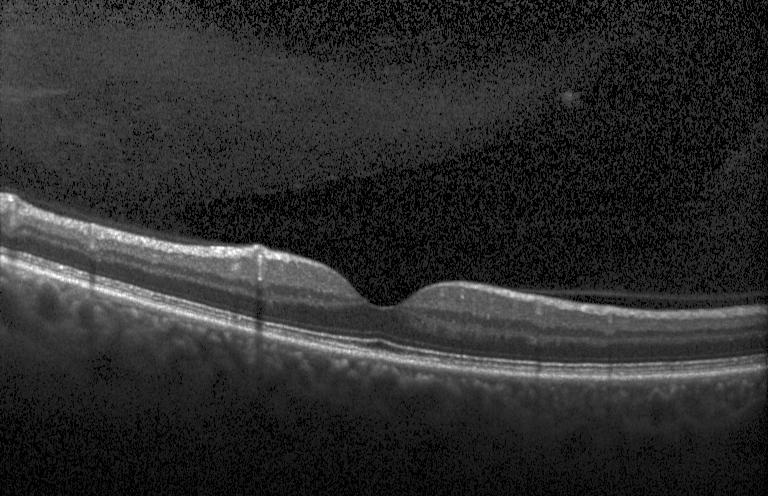 Heidelberg Spectralis OCT system · SD-OCT · OCT B-scan
Assessment: neither choroidal neovascularization, diabetic macular edema, nor drusen.